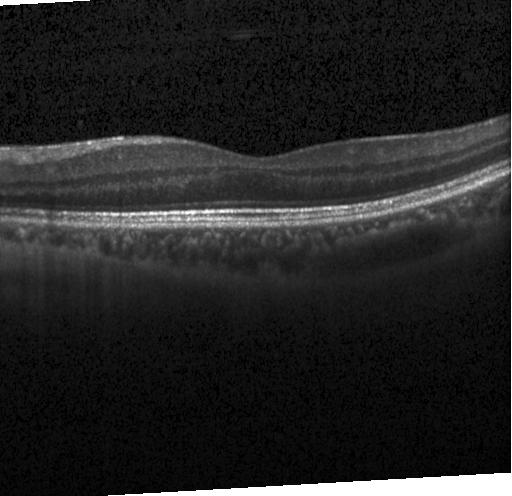 Macular OCT demonstrating no evidence of choroidal neovascularization, diabetic macular edema, or drusen.